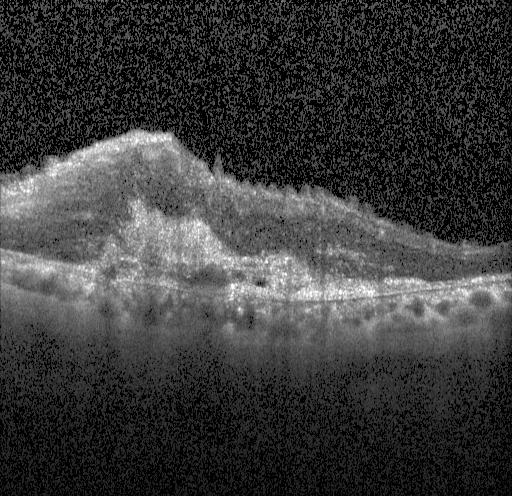
Optical coherence tomography B-scan
Assessment: a choroidal neovascular membrane.